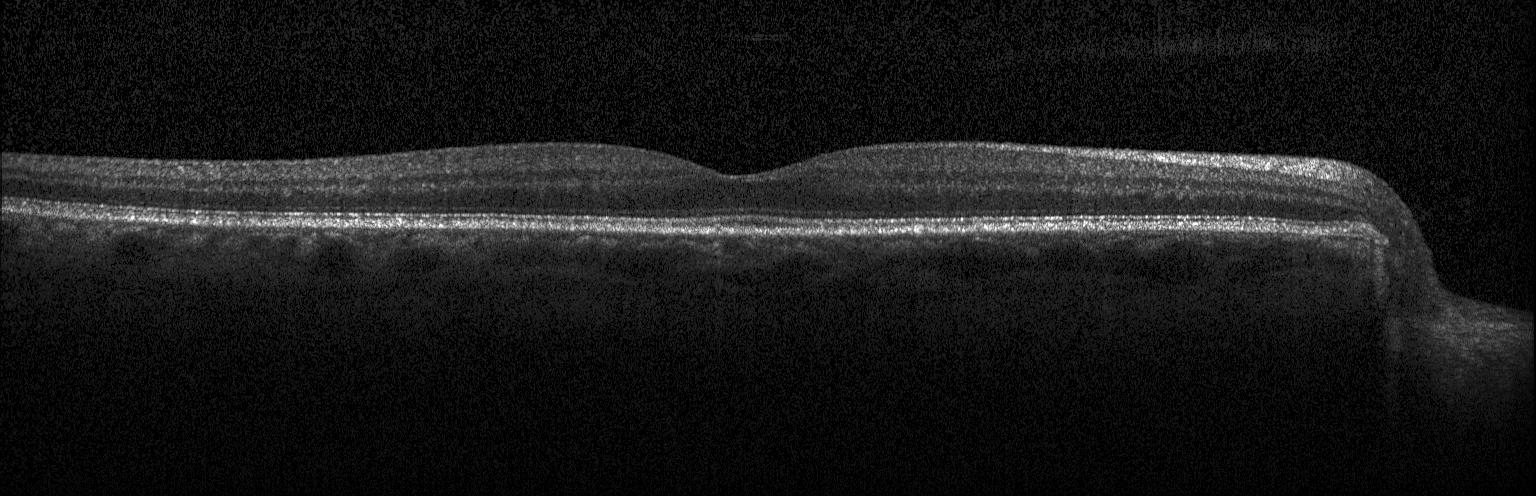

Dx: no CNV, DME, or drusen.